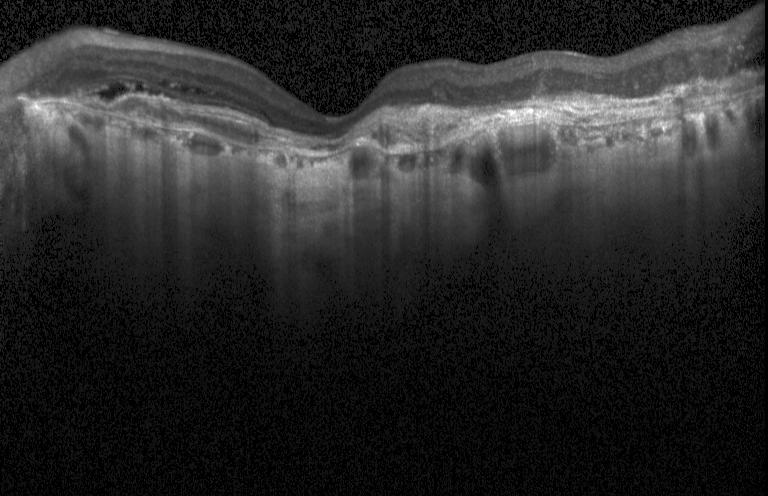
Impression: a choroidal neovascular membrane.